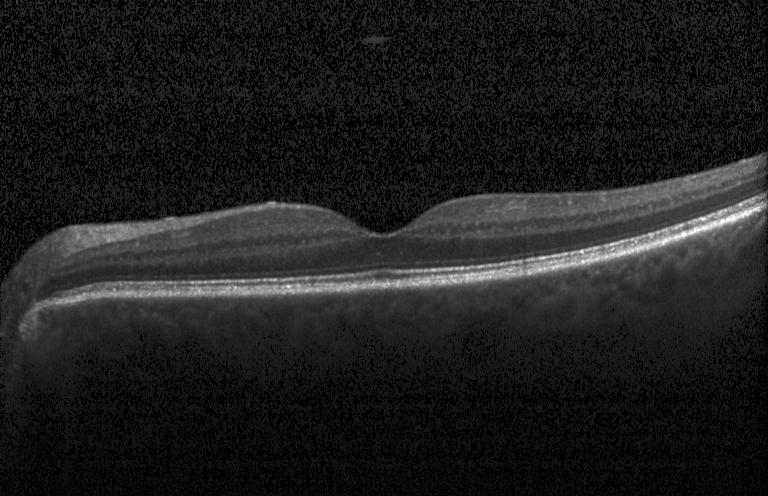 OCT scan showing no choroidal neovascularization, no diabetic macular edema, and no drusen.